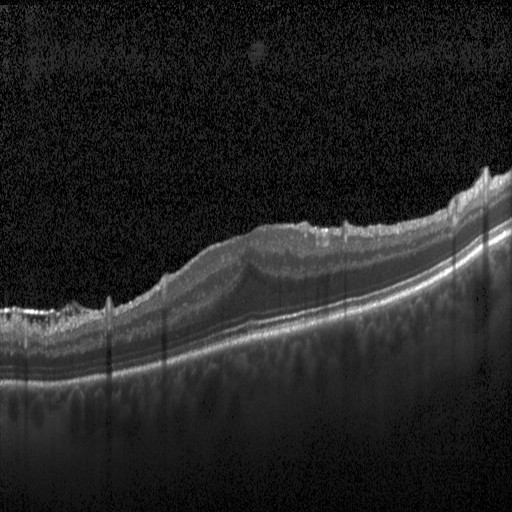

Dx: diabetic macular edema.